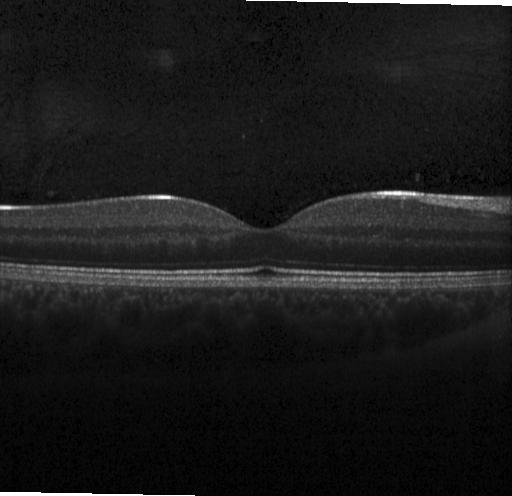 OCT finding: no choroidal neovascularization, no diabetic macular edema, and no drusen.